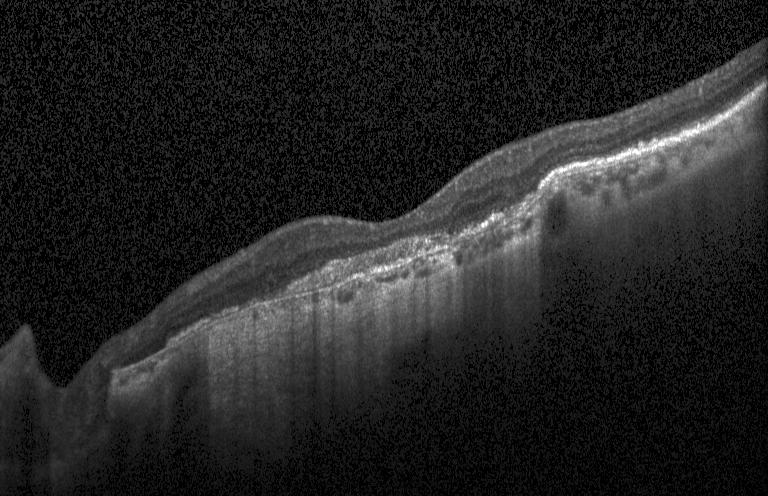
OCT B-scan. Spectral-domain optical coherence tomography
The scan shows choroidal neovascularization.